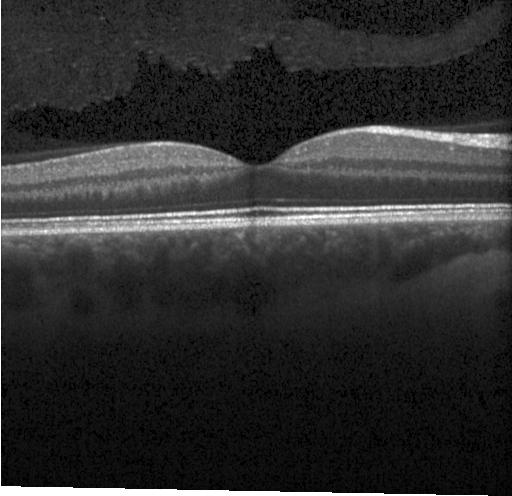 Centered on the fovea; Heidelberg Spectralis; optical coherence tomography scan; spectral-domain OCT — Impression: neither choroidal neovascularization, diabetic macular edema, nor drusen.